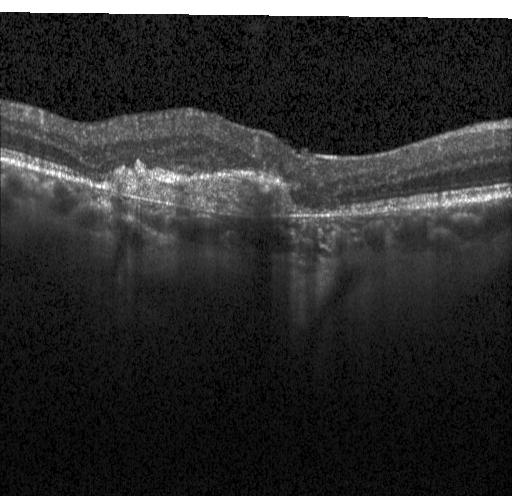
OCT finding: CNV.